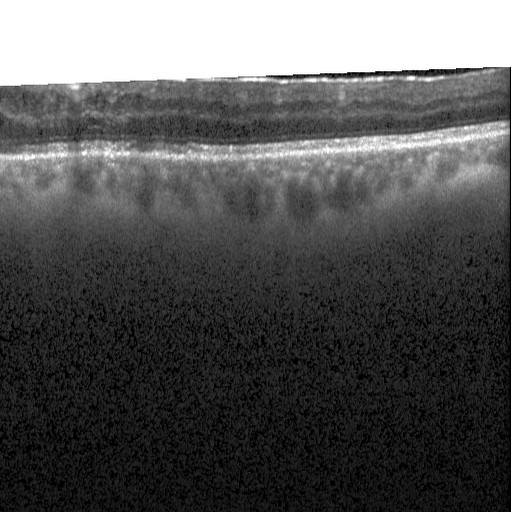
DME.